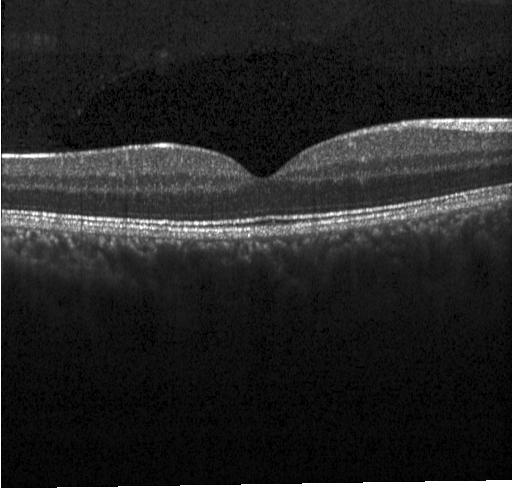

Impression: no choroidal neovascularization, diabetic macular edema, or drusen.